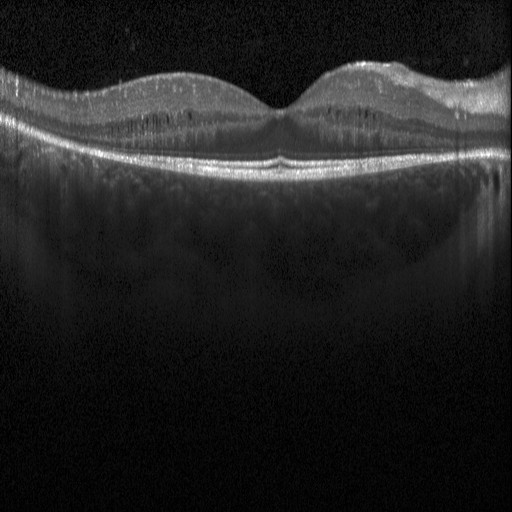
OCT scan showing diabetic macular edema (DME).